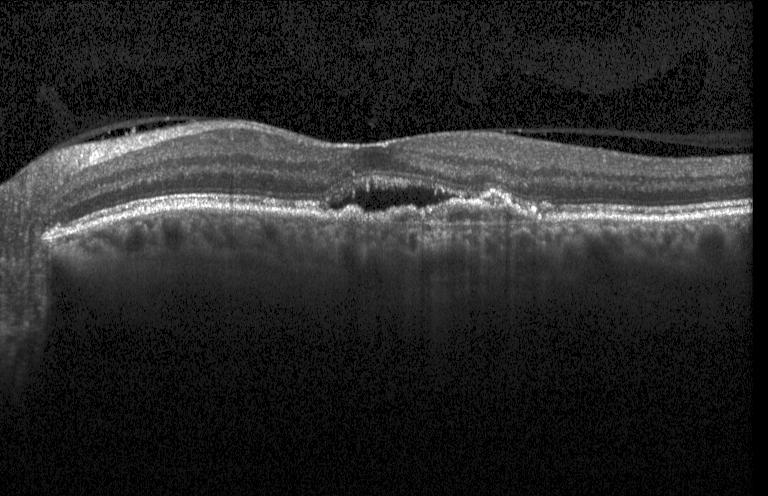

Impression: choroidal neovascularization.